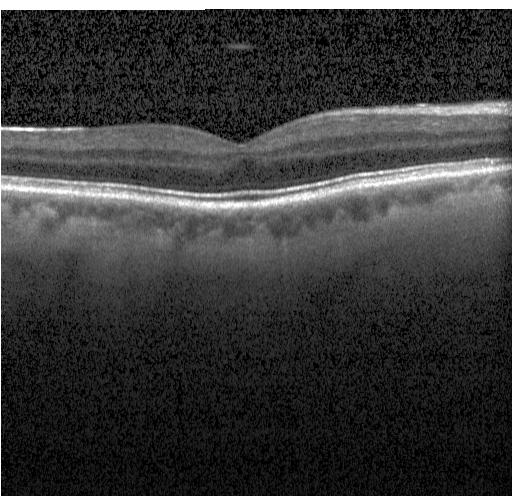

Optical coherence tomography scan · spectral-domain optical coherence tomography.
Finding: no choroidal neovascularization, diabetic macular edema, or drusen.